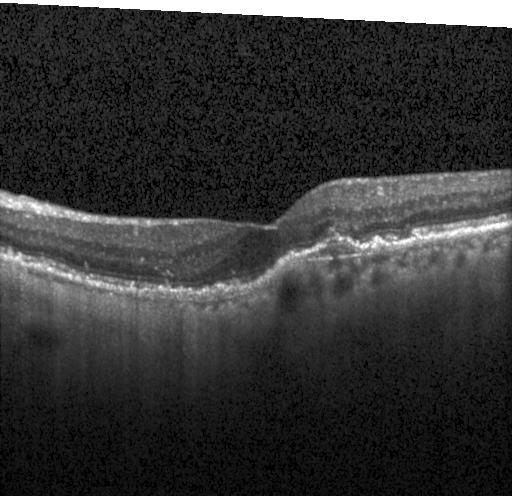
Horizontal scan through the fovea; spectral-domain OCT; OCT line scan; Heidelberg Spectralis OCT system.
Choroidal neovascularization.